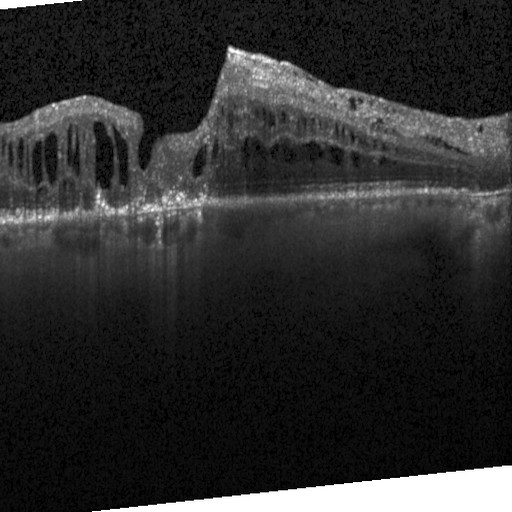
Diagnosis: diabetic macular edema.